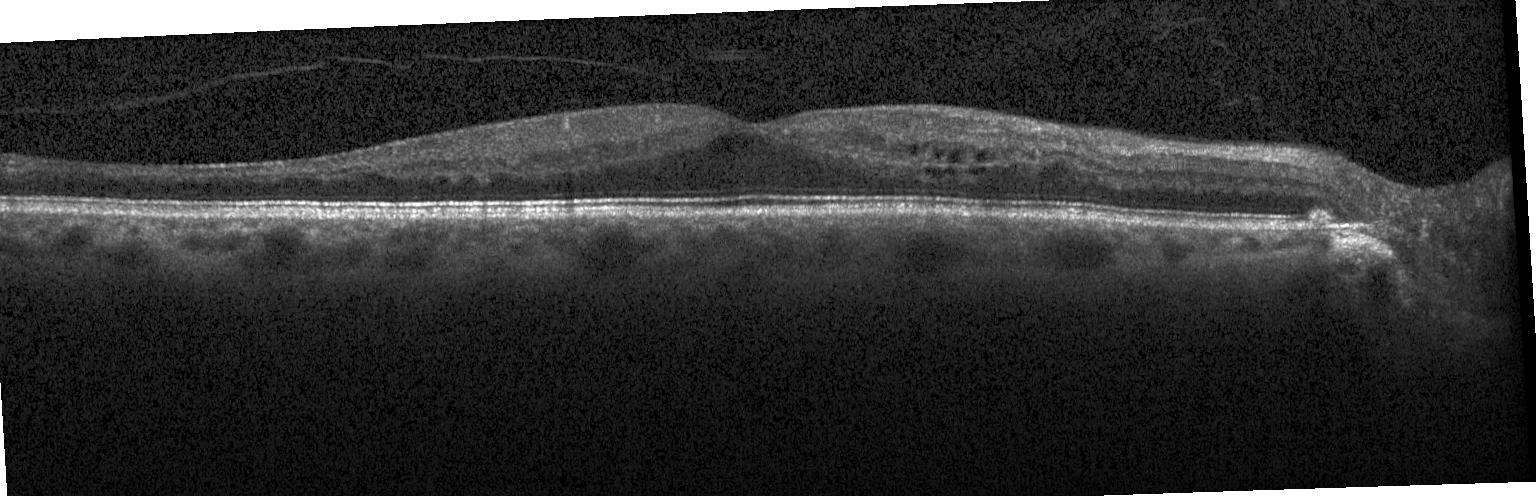
Centered on the fovea. OCT B-scan. Heidelberg Spectralis OCT system. Assessment: diabetic macular edema.